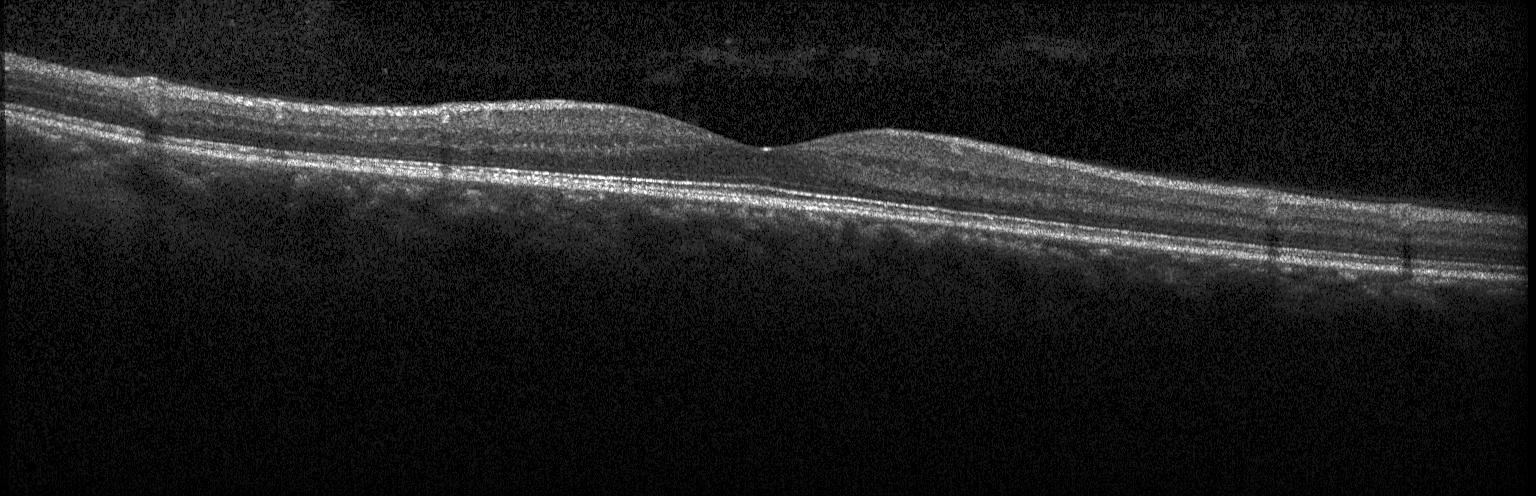

Fovea-centered · spectral-domain OCT · instrument: Heidelberg Spectralis · retinal OCT cross-section
OCT finding: no evidence of CNV, DME, or drusen.